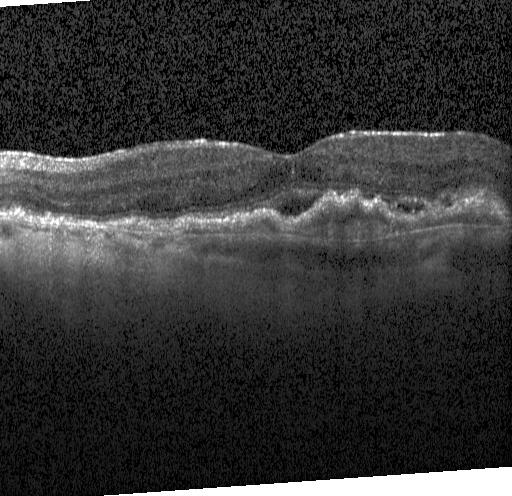
Assessment: choroidal neovascularization (CNV).